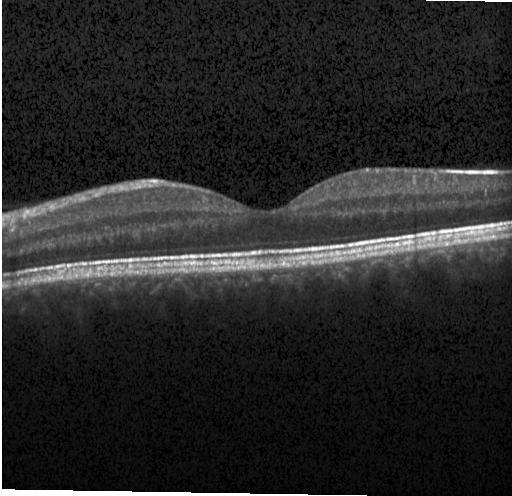
OCT B-scan — Dx: no choroidal neovascularization, no diabetic macular edema, and no drusen.